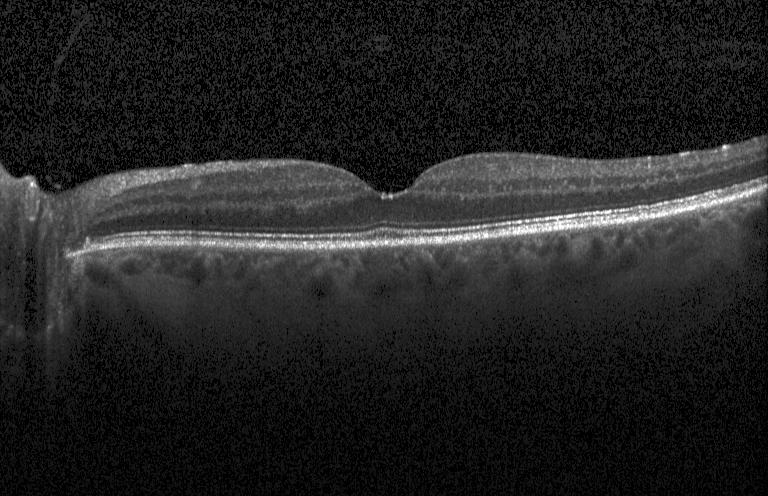 Optical coherence tomography scan, horizontal scan through the fovea, instrument: Heidelberg Spectralis
No evidence of choroidal neovascularization, diabetic macular edema, or drusen.